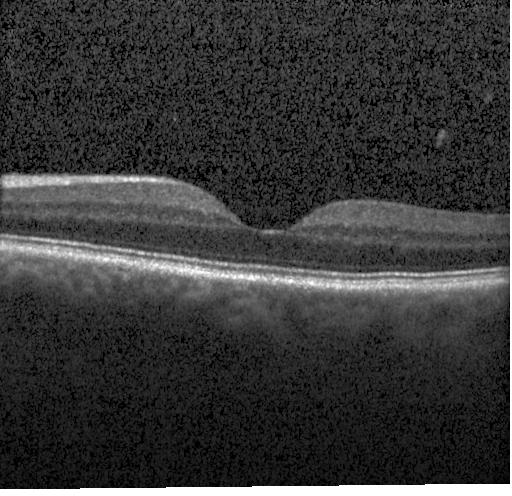

Optical coherence tomography scan, horizontal scan through the fovea. Impression: neither CNV, DME, nor drusen.